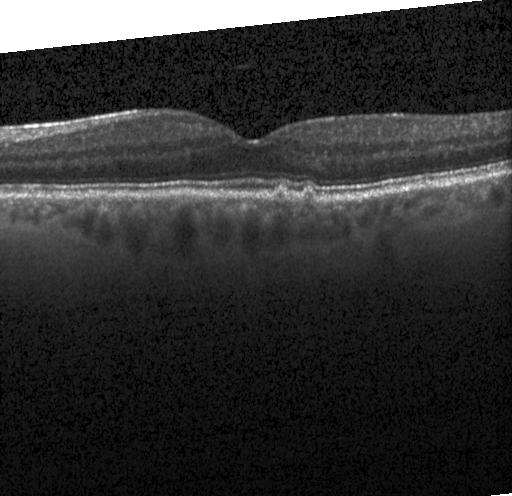

Macular OCT demonstrating sub-RPE drusenoid deposits.